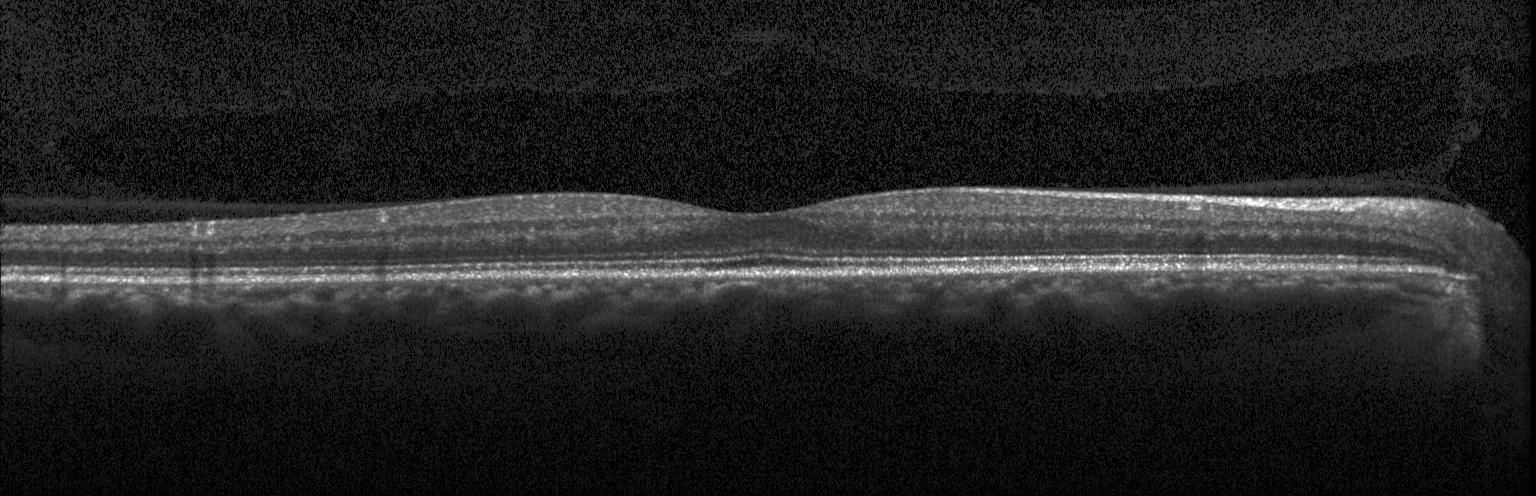

Retinal OCT cross-section showing no evidence of choroidal neovascularization, diabetic macular edema, or drusen.